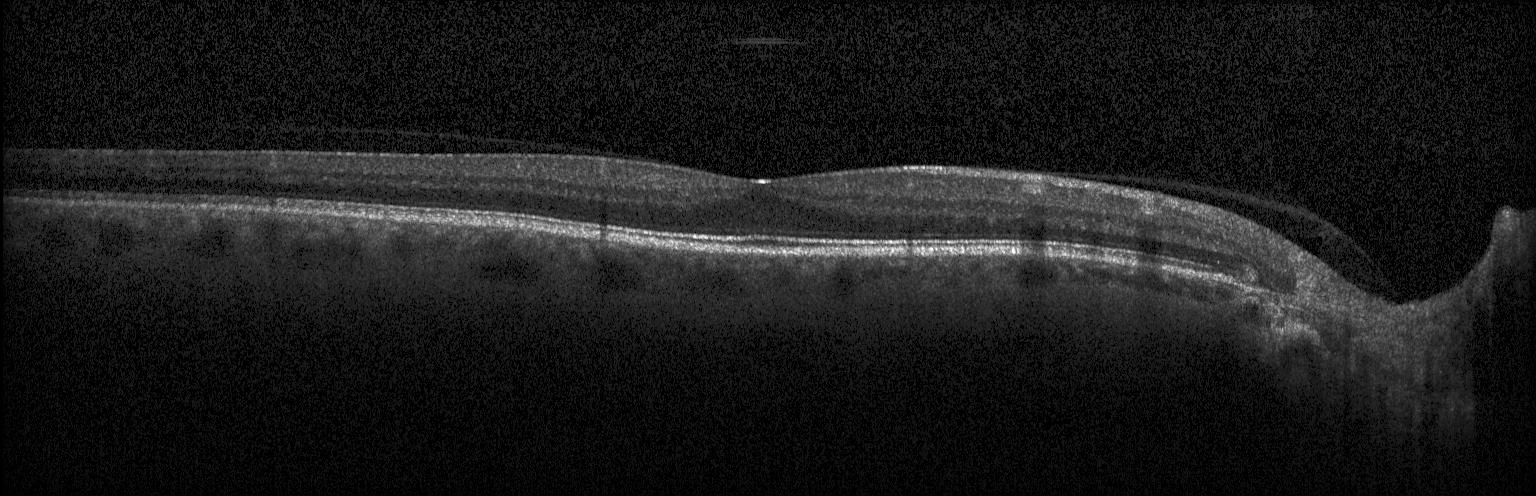
Retinal OCT cross-section; Heidelberg Spectralis OCT system; through the macula; spectral-domain optical coherence tomography. This B-scan demonstrates no evidence of CNV, DME, or drusen.